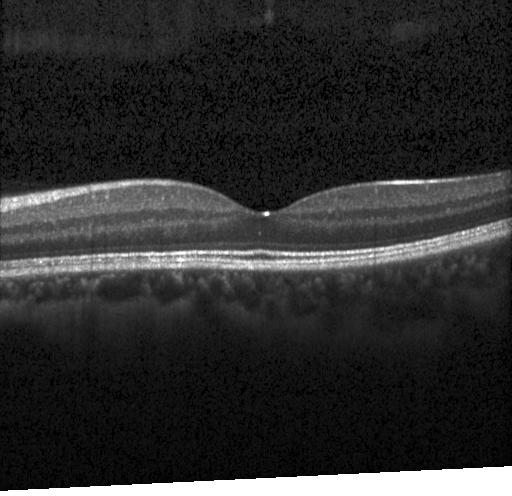
Macular OCT demonstrating neither choroidal neovascularization, diabetic macular edema, nor drusen.